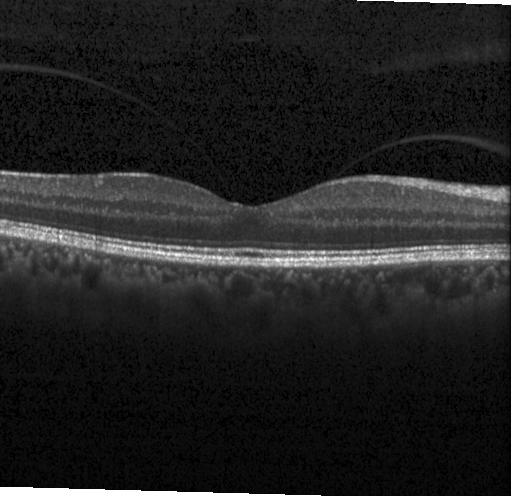
Spectral-domain OCT. Retinal OCT B-scan. Through the macula.
Finding: no choroidal neovascularization, diabetic macular edema, or drusen.